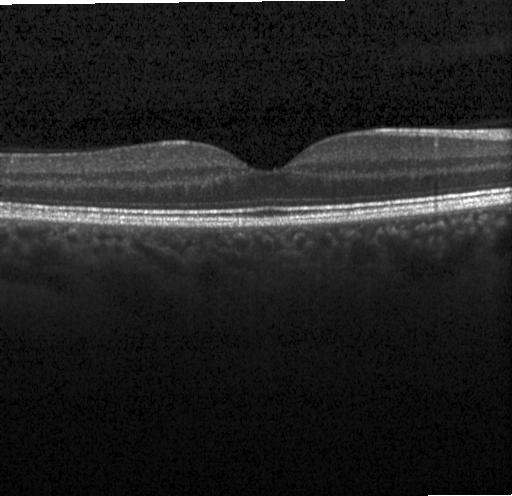

Macular scan, SD-OCT, retinal OCT B-scan.
OCT finding: no choroidal neovascularization, diabetic macular edema, or drusen.